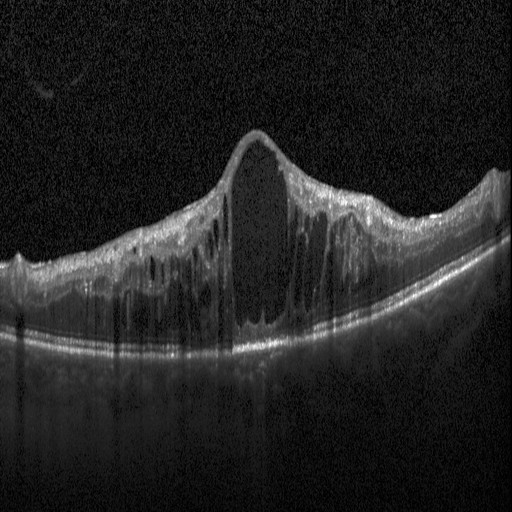

OCT line scan. Impression: diabetic macular edema.